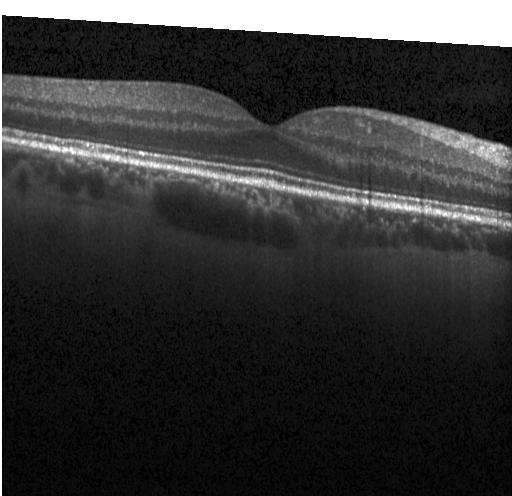
Through the macula · retinal OCT cross-section — The scan shows no evidence of choroidal neovascularization, diabetic macular edema, or drusen.